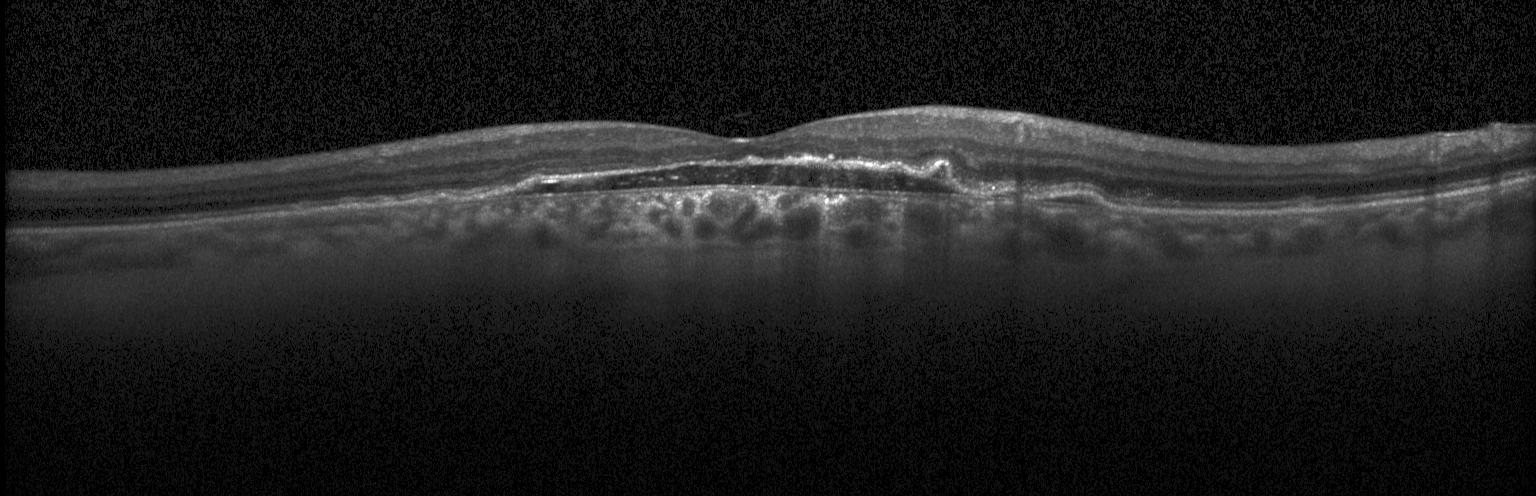 Spectral-domain OCT B-scan: a choroidal neovascular membrane.